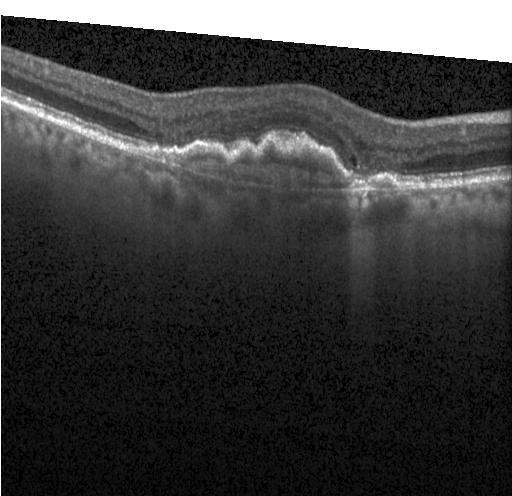 Optical coherence tomography scan, macular scan, Heidelberg Spectralis
The scan shows choroidal neovascularization (CNV).